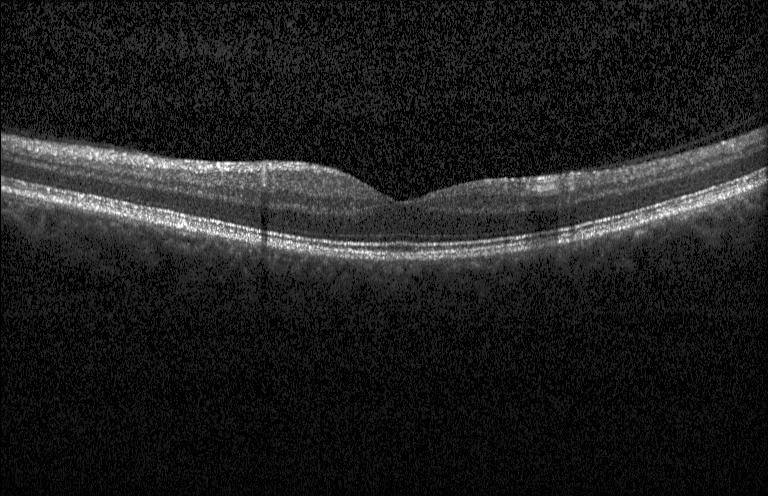 Assessment: no CNV, DME, or drusen.